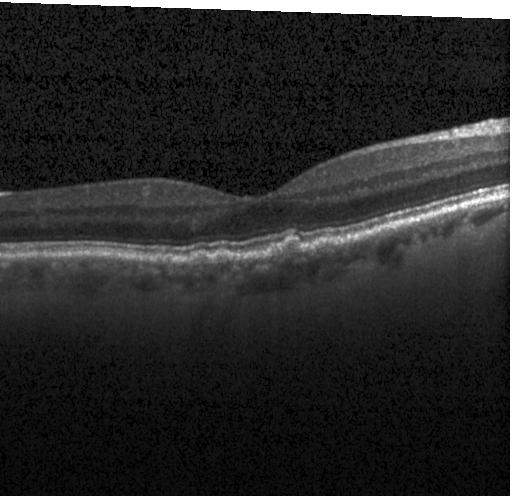
Spectral-domain OCT B-scan: sub-RPE drusenoid deposits.